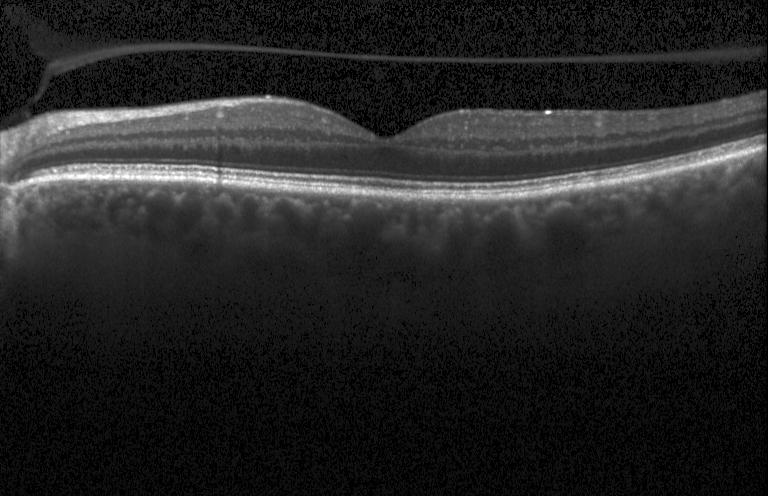

Impression: no choroidal neovascularization, no diabetic macular edema, and no drusen.